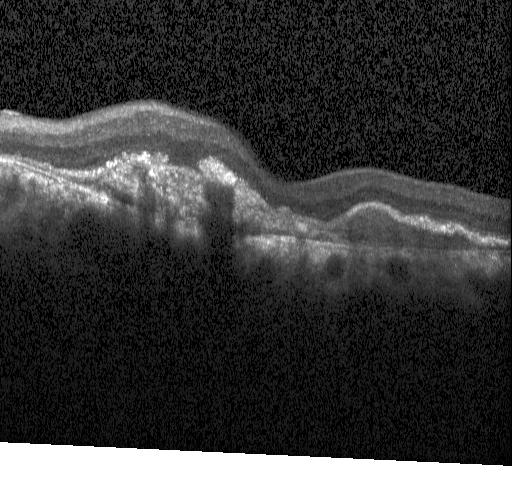

OCT B-scan; spectral-domain optical coherence tomography; Heidelberg Spectralis; horizontal scan through the fovea — Assessment: choroidal neovascularization (CNV).